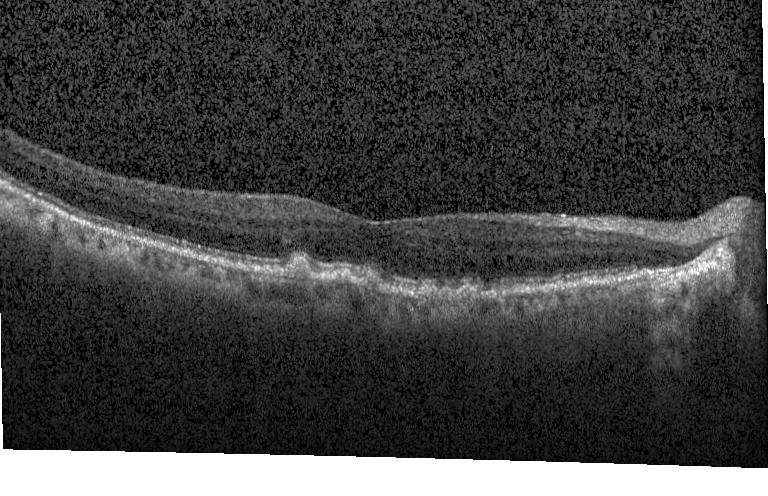

Spectral-domain optical coherence tomography. Macular scan. OCT line scan. Acquired on a Heidelberg Spectralis — Diagnosis: sub-RPE drusenoid deposits.